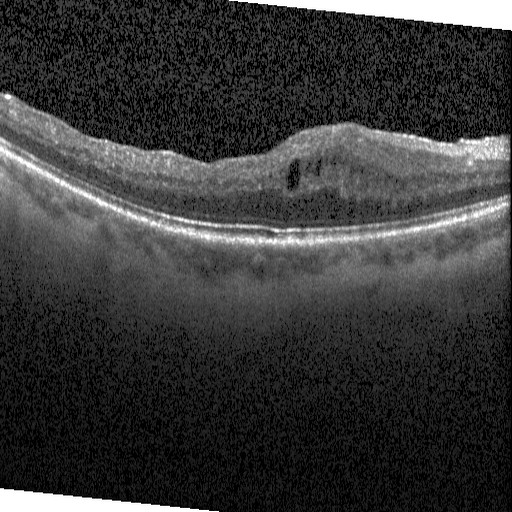

Retinal OCT cross-section
Finding: diabetic macular edema (DME).